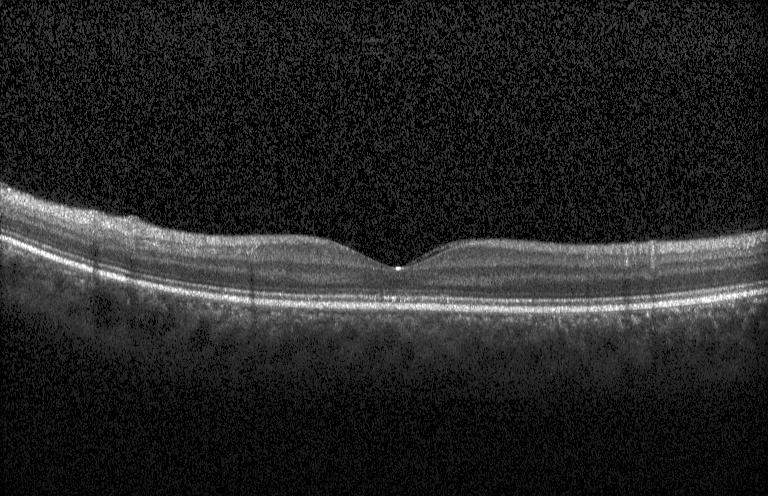
OCT B-scan
The scan shows neither choroidal neovascularization, diabetic macular edema, nor drusen.